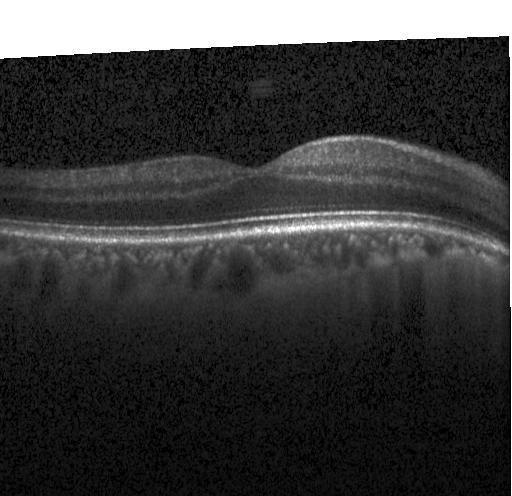

Fovea-centered, OCT B-scan, SD-OCT, instrument: Heidelberg Spectralis. Finding: neither choroidal neovascularization, diabetic macular edema, nor drusen.